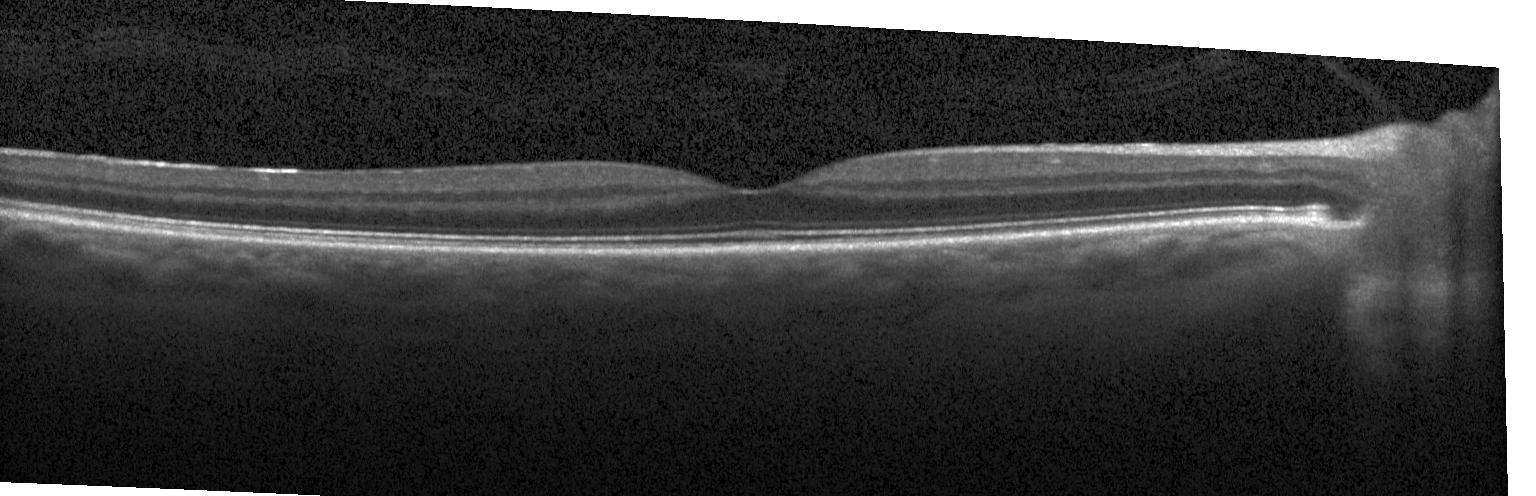

SD-OCT, centered on the fovea, optical coherence tomography B-scan
Impression: no choroidal neovascularization, diabetic macular edema, or drusen.